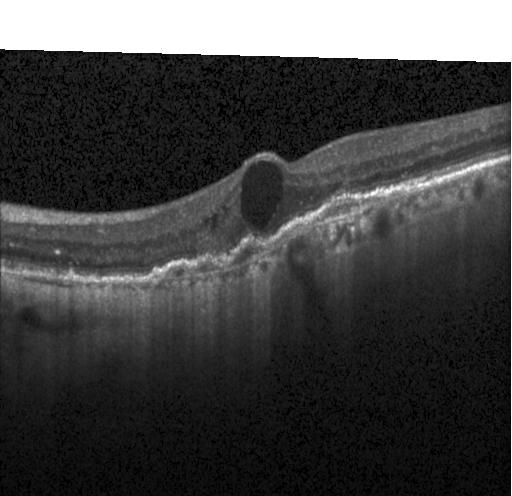 Impression: a choroidal neovascular membrane.